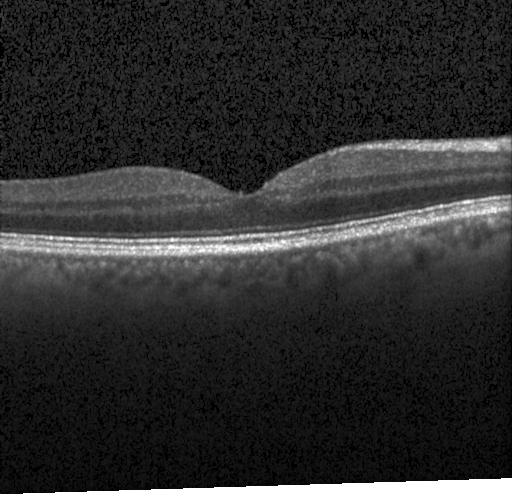
Horizontal scan through the fovea, instrument: Heidelberg Spectralis, OCT B-scan — This B-scan demonstrates neither CNV, DME, nor drusen.